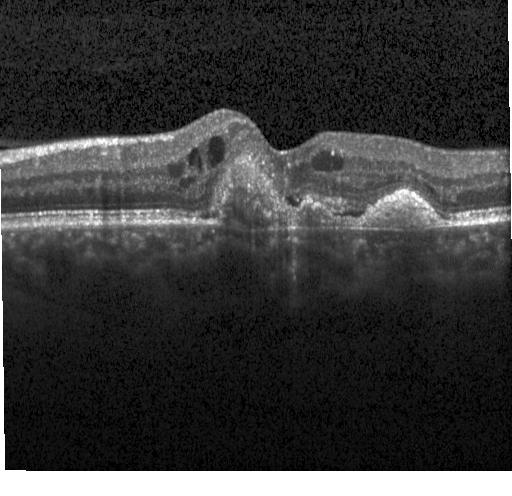
Diagnosis: a choroidal neovascular membrane.